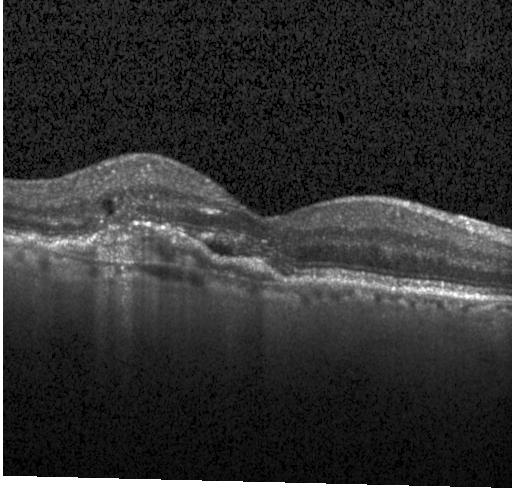 Assessment: a choroidal neovascular membrane.